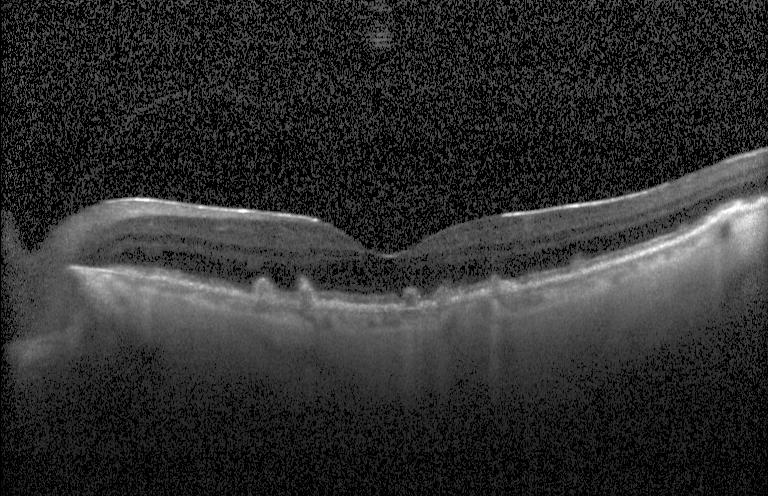 OCT B-scan showing drusen.